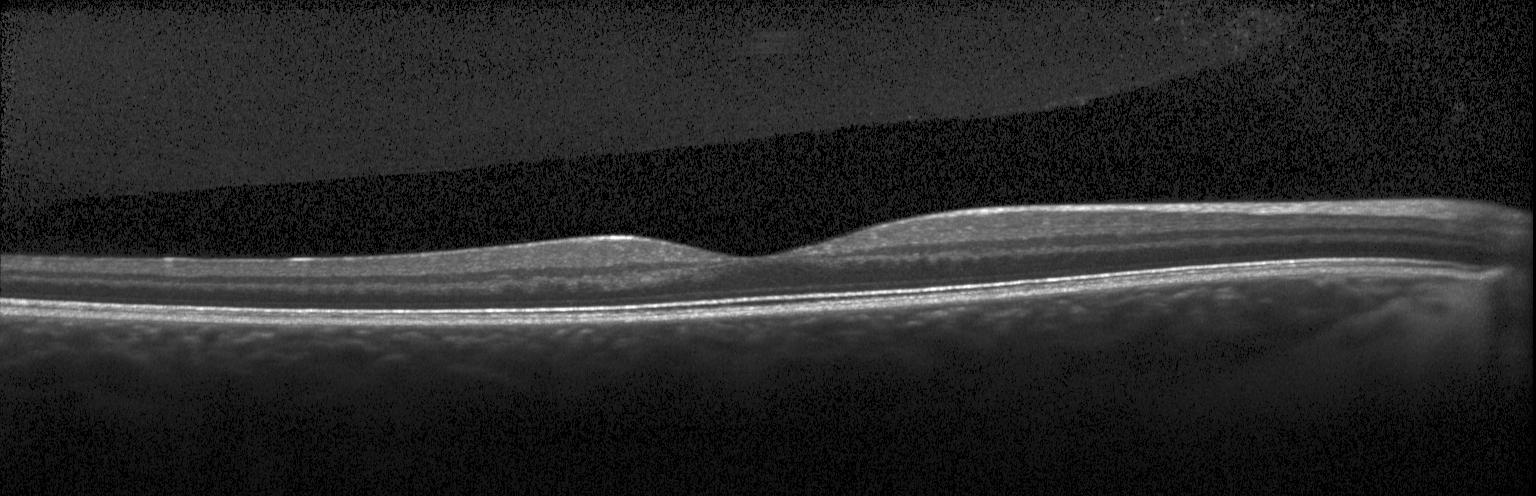
OCT line scan · spectral-domain optical coherence tomography · acquired on a Heidelberg Spectralis · horizontal scan through the fovea.
Assessment: no choroidal neovascularization, no diabetic macular edema, and no drusen.